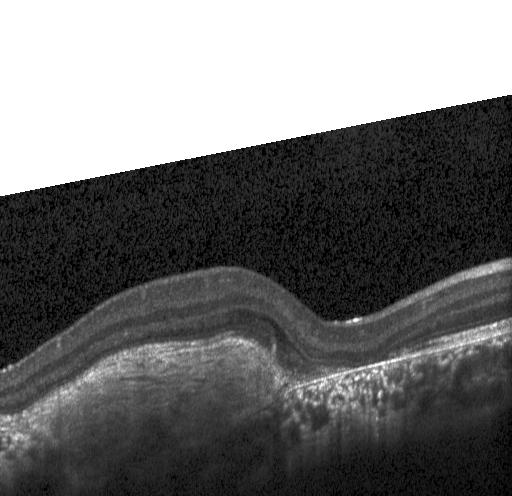 Spectral-domain optical coherence tomography · horizontal scan through the fovea · optical coherence tomography B-scan · instrument: Heidelberg Spectralis
A choroidal neovascular membrane.